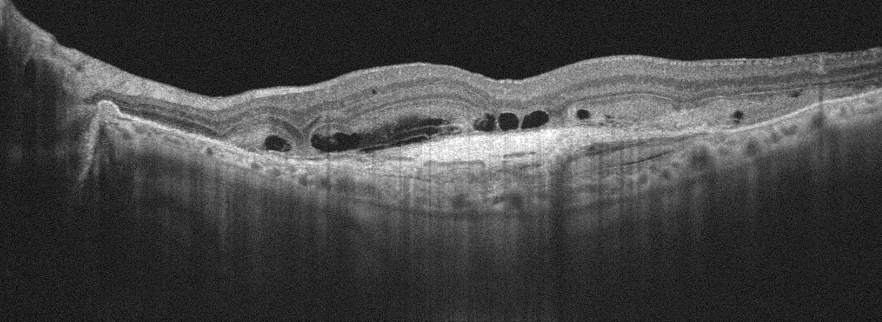
OCT B-scan — Macular OCT: age-related macular degeneration (AMD).